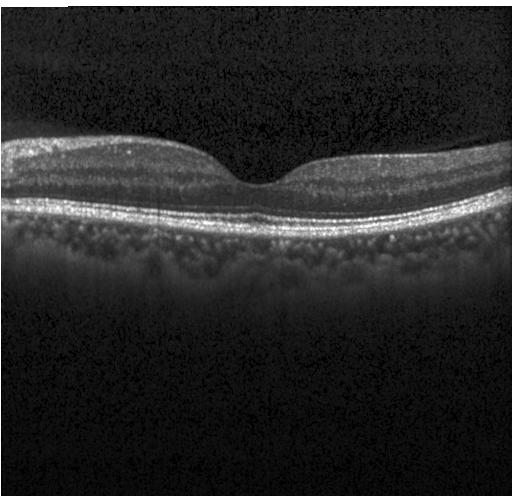

Fovea-centered; optical coherence tomography B-scan; SD-OCT.
Finding: neither choroidal neovascularization, diabetic macular edema, nor drusen.